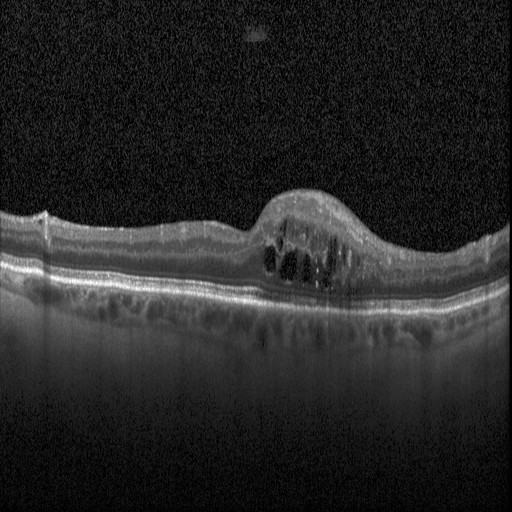
Assessment: diabetic macular edema.